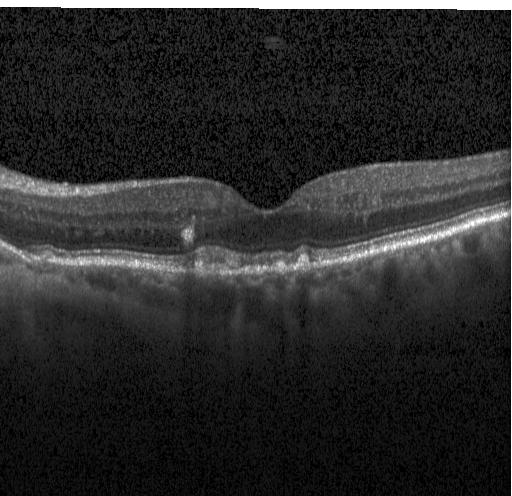 OCT B-scan showing sub-RPE drusenoid deposits.